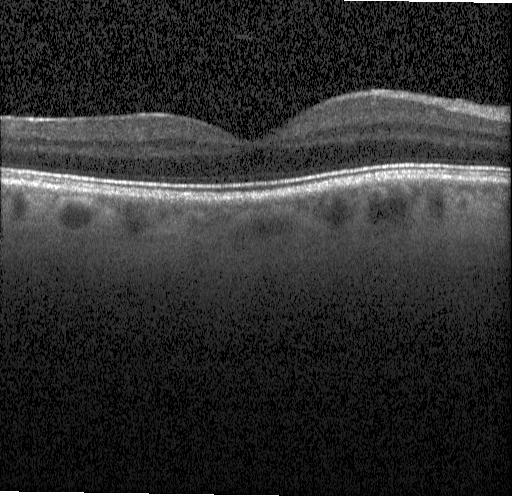

Diagnosis: no choroidal neovascularization, diabetic macular edema, or drusen.